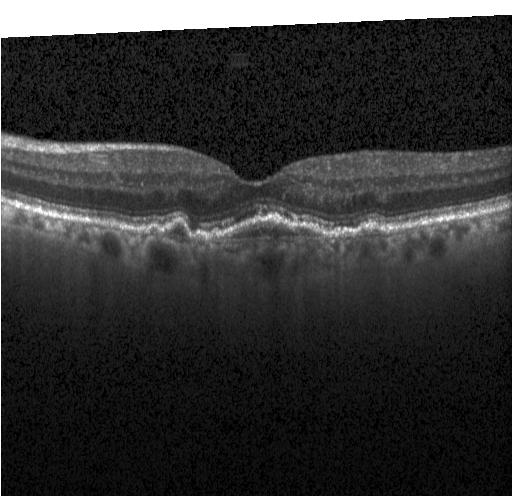
Optical coherence tomography scan.
Finding: choroidal neovascularization (CNV).